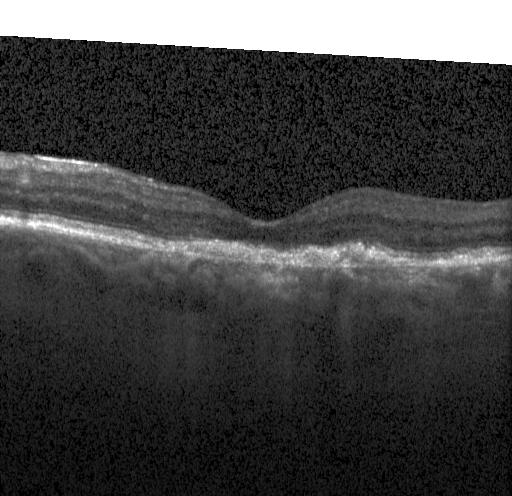
Heidelberg Spectralis OCT system, retinal OCT cross-section.
Choroidal neovascularization.